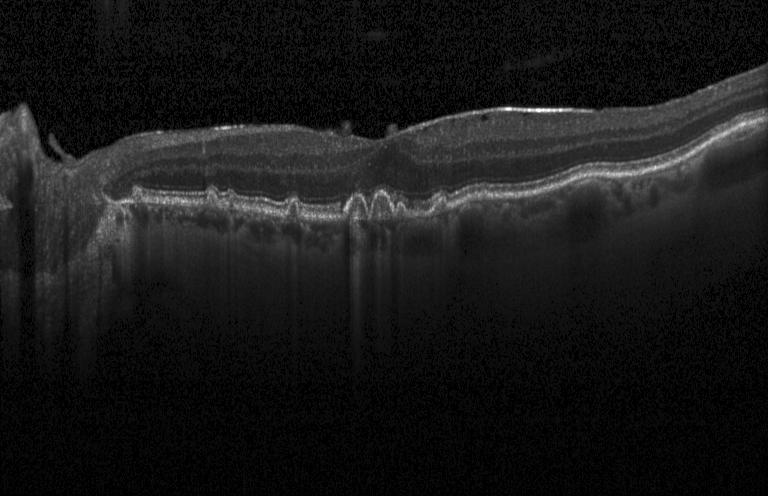
OCT scan showing sub-RPE drusenoid deposits.